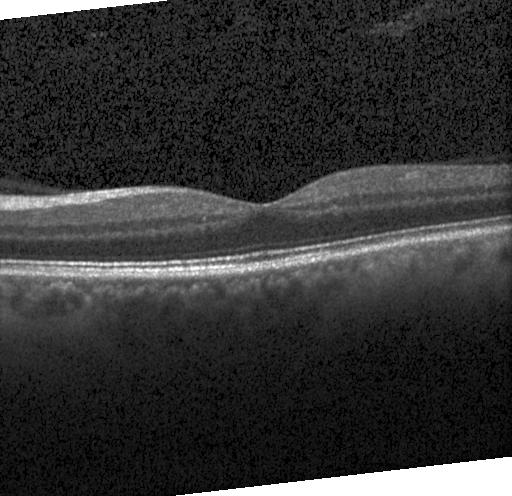

Diagnosis: no choroidal neovascularization, no diabetic macular edema, and no drusen.